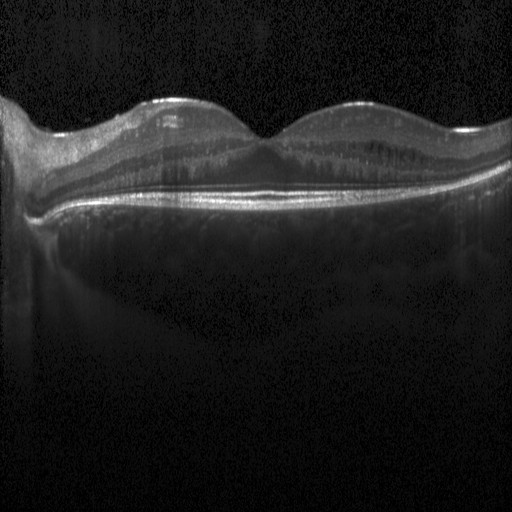

OCT scan showing diabetic macular edema.